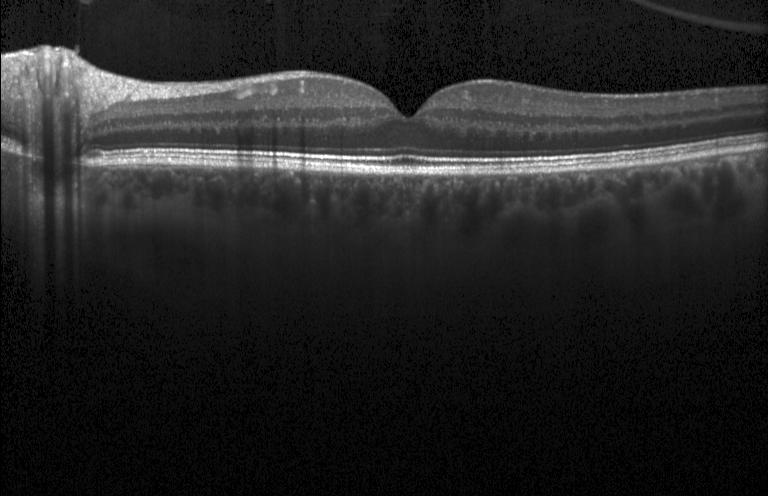
Impression: no evidence of choroidal neovascularization, diabetic macular edema, or drusen.